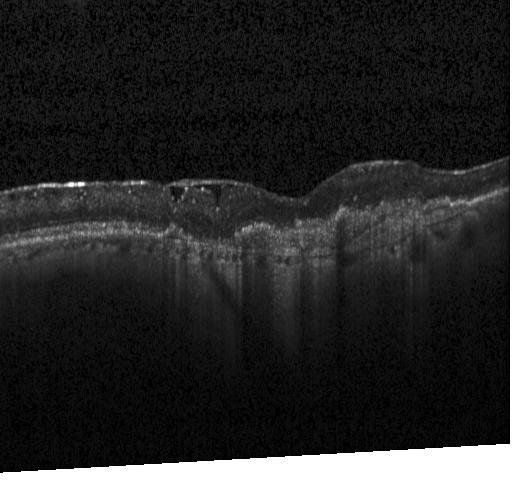 Dx: choroidal neovascularization.